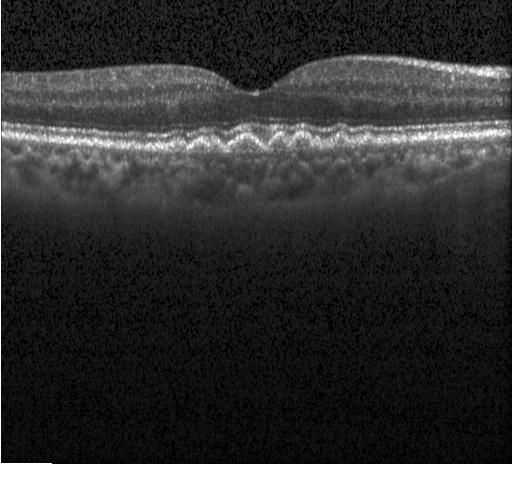

Optical coherence tomography scan. Spectral-domain optical coherence tomography. Heidelberg Spectralis
OCT finding: sub-RPE drusenoid deposits.